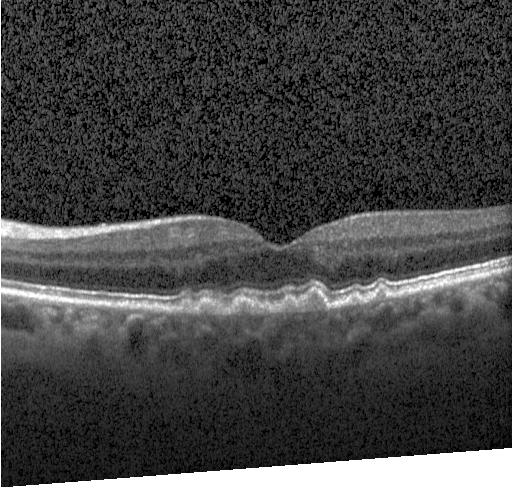

Horizontal scan through the fovea. OCT B-scan — Finding: multiple drusen.